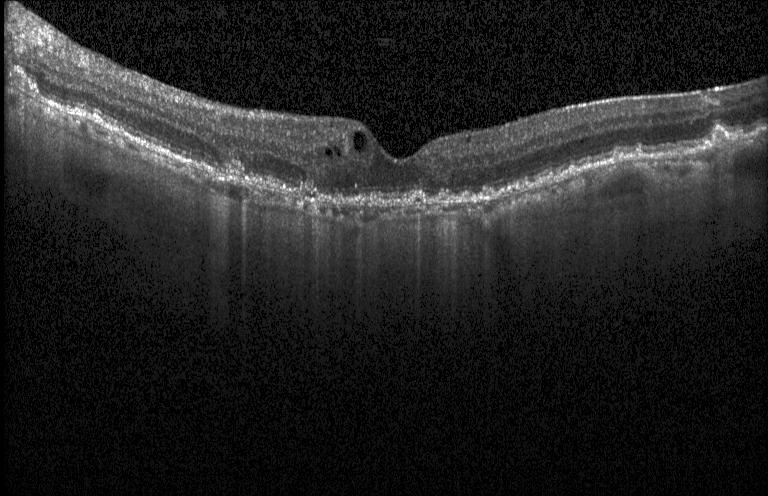

Retinal OCT B-scan — Macular OCT: a choroidal neovascular membrane.